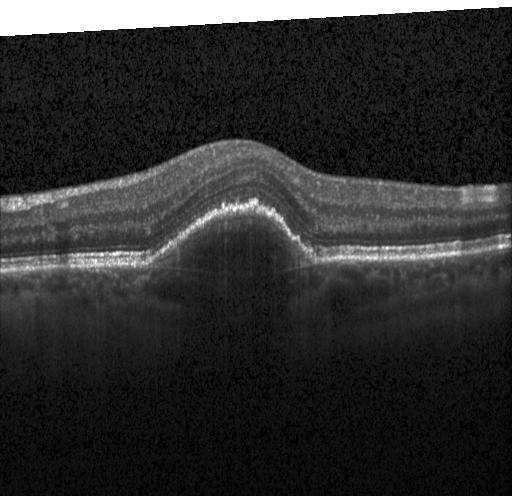 Macular OCT demonstrating a choroidal neovascular membrane.